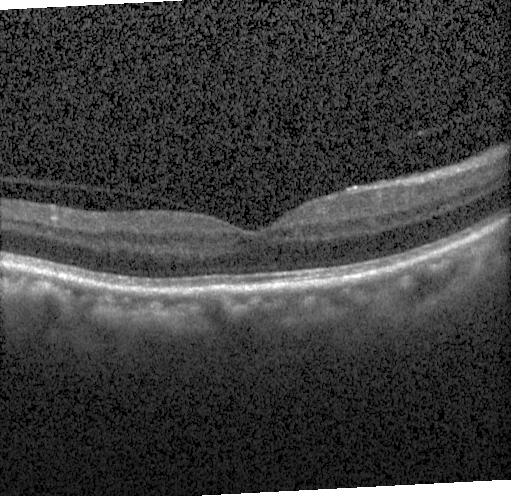
Retinal OCT B-scan
Diagnosis: no choroidal neovascularization, no diabetic macular edema, and no drusen.